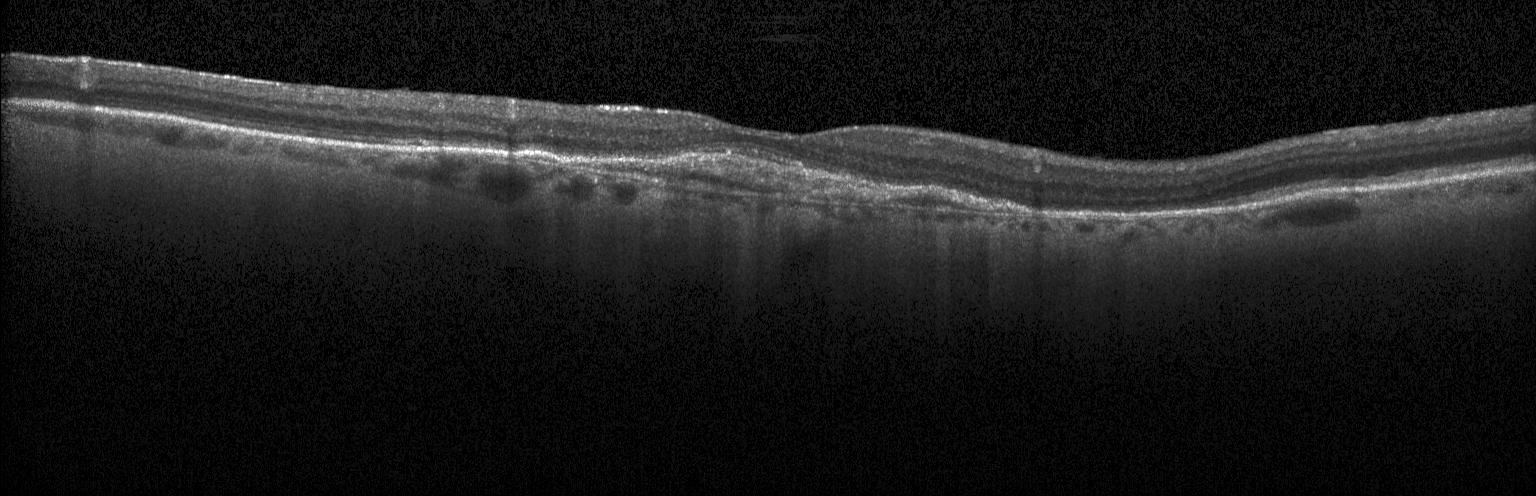

Centered on the fovea · retinal OCT B-scan · spectral-domain optical coherence tomography · Heidelberg Spectralis OCT system — Choroidal neovascularization (CNV).